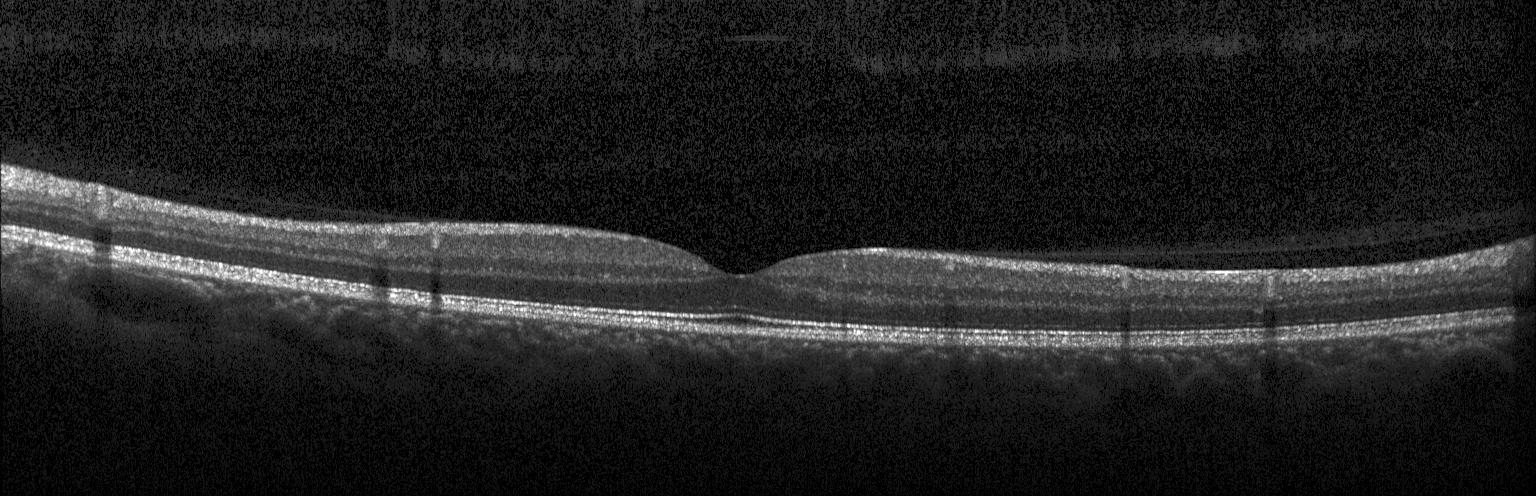 Spectral-domain optical coherence tomography; OCT B-scan; instrument: Heidelberg Spectralis.
Finding: no evidence of choroidal neovascularization, diabetic macular edema, or drusen.